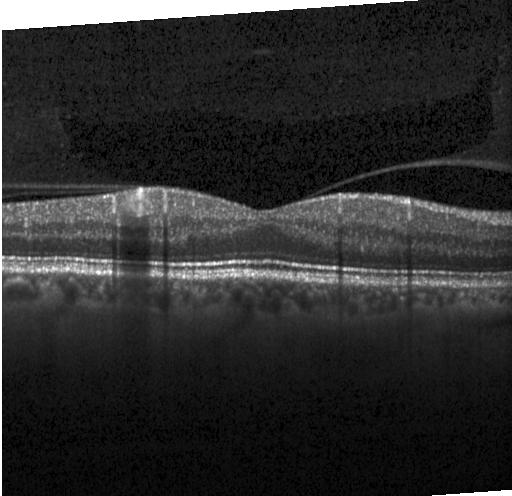 SD-OCT, Heidelberg Spectralis OCT system, OCT B-scan — Neither choroidal neovascularization, diabetic macular edema, nor drusen.